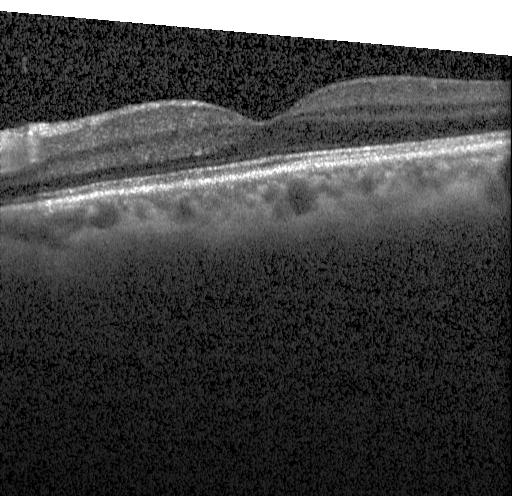
Diagnosis: no evidence of CNV, DME, or drusen.